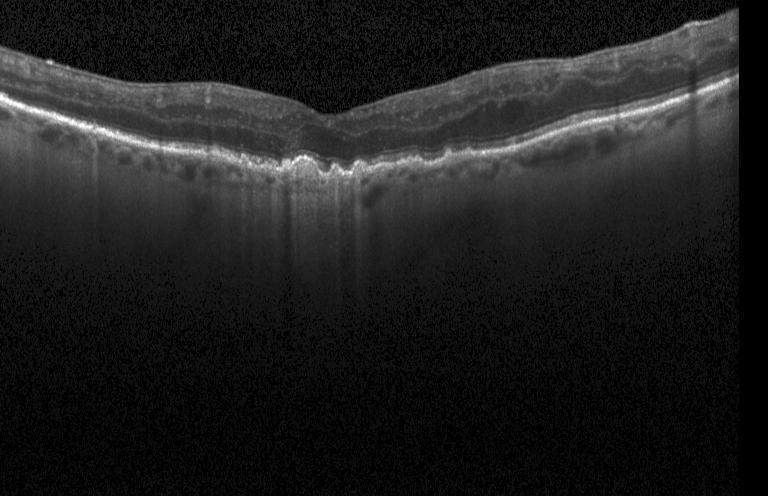

Optical coherence tomography scan — Finding: CNV.